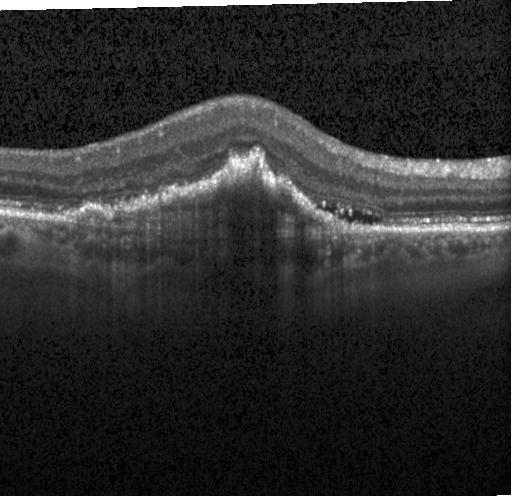 Optical coherence tomography B-scan; spectral-domain optical coherence tomography.
Assessment: choroidal neovascularization.